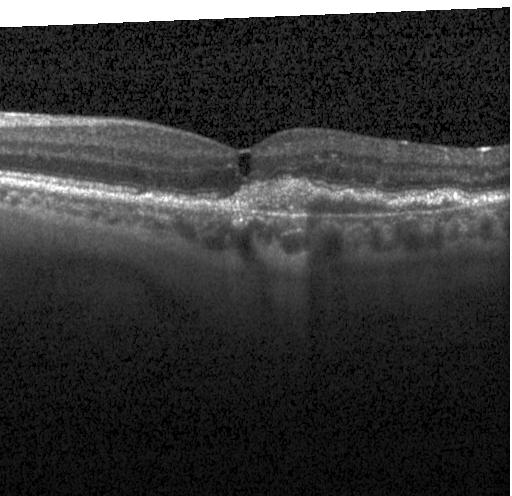

Centered on the fovea. Optical coherence tomography B-scan.
Macular OCT: CNV.